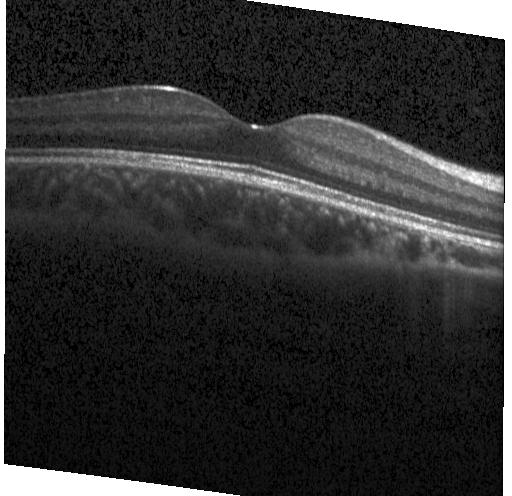
OCT line scan — Impression: no choroidal neovascularization, no diabetic macular edema, and no drusen.